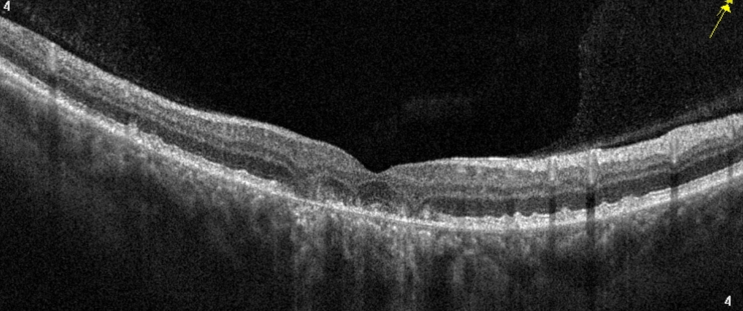 OCT scan showing age-related macular degeneration (AMD).